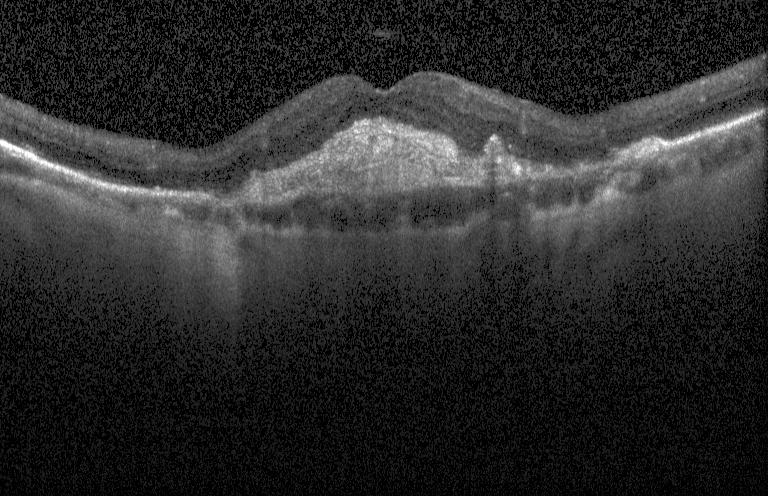
Acquired on a Heidelberg Spectralis. Fovea-centered. OCT line scan. Spectral-domain optical coherence tomography — Impression: a choroidal neovascular membrane.